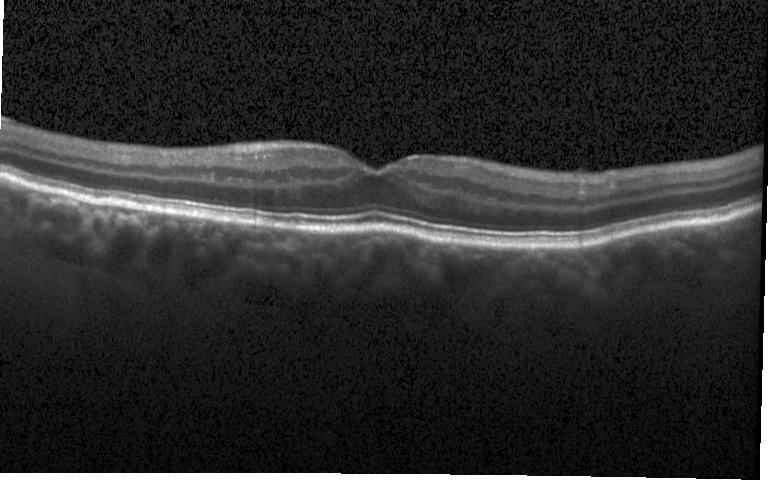
Dx: no choroidal neovascularization, no diabetic macular edema, and no drusen.